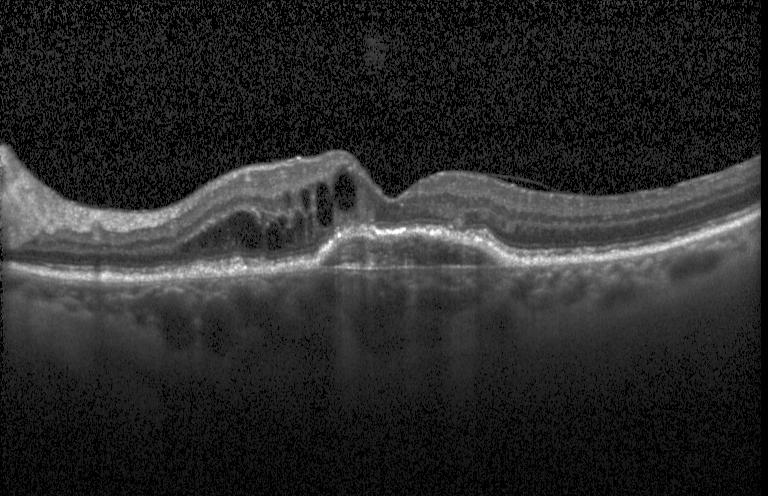

Spectral-domain OCT, retinal OCT B-scan, acquired on a Heidelberg Spectralis — Diagnosis: a choroidal neovascular membrane.